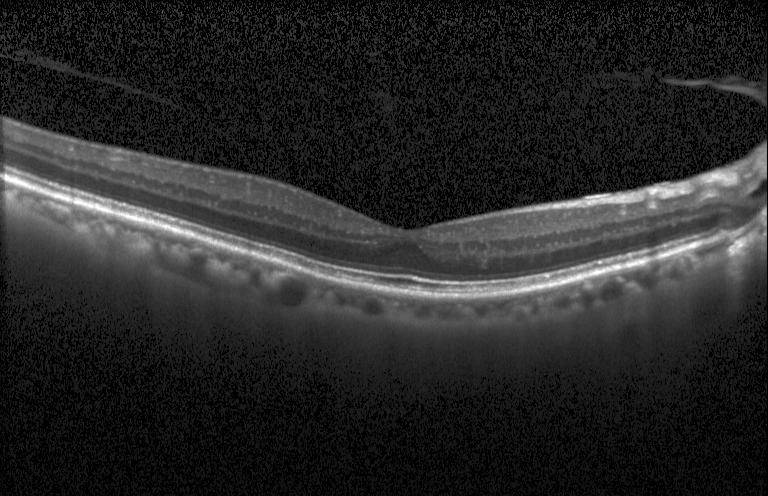 Heidelberg Spectralis, horizontal scan through the fovea, retinal OCT cross-section — Diagnosis: no evidence of choroidal neovascularization, diabetic macular edema, or drusen.